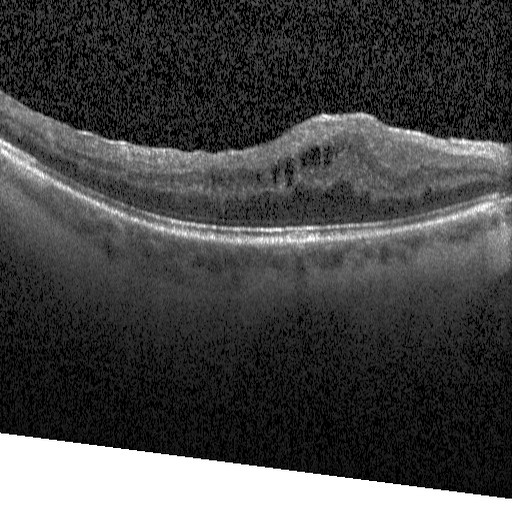

DME.